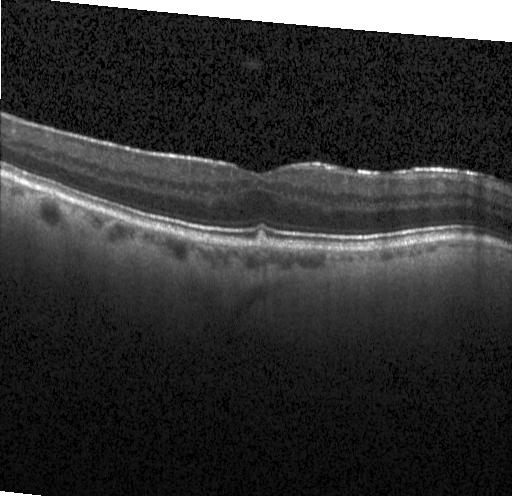 OCT line scan
Finding: sub-RPE drusenoid deposits.